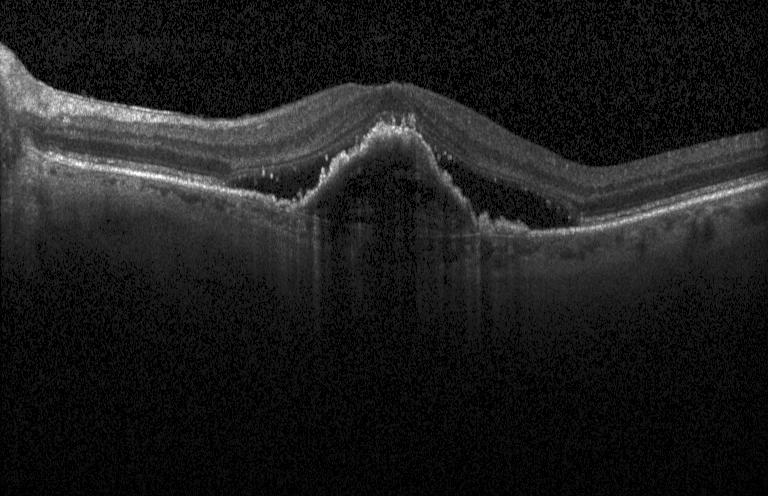

Optical coherence tomography B-scan. Through the macula — Impression: choroidal neovascularization.